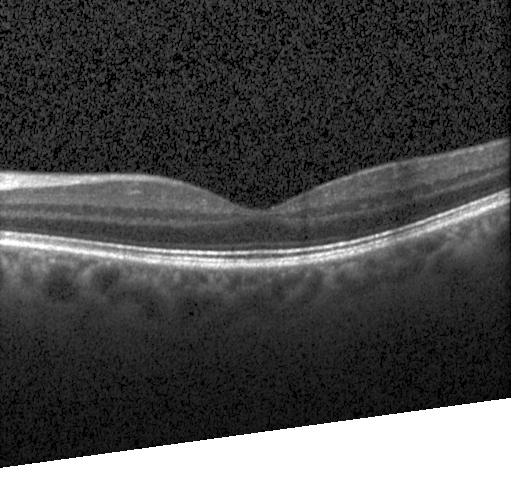

OCT B-scan, macular scan, Heidelberg Spectralis OCT system — Dx: neither choroidal neovascularization, diabetic macular edema, nor drusen.